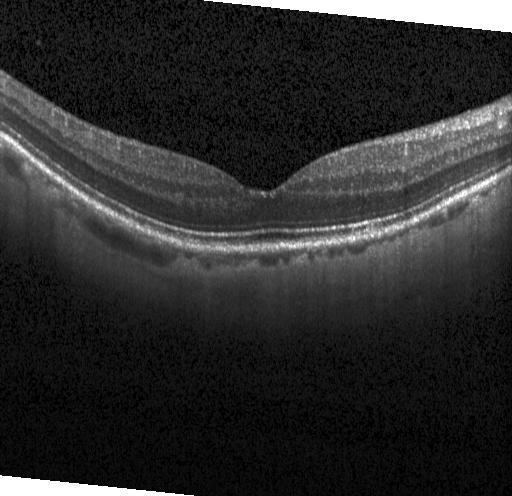
Macular OCT: neither choroidal neovascularization, diabetic macular edema, nor drusen.